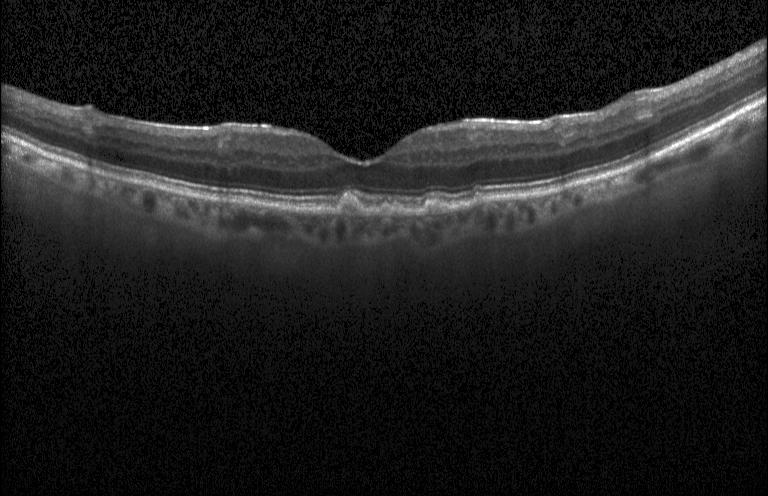
Finding: multiple drusen.